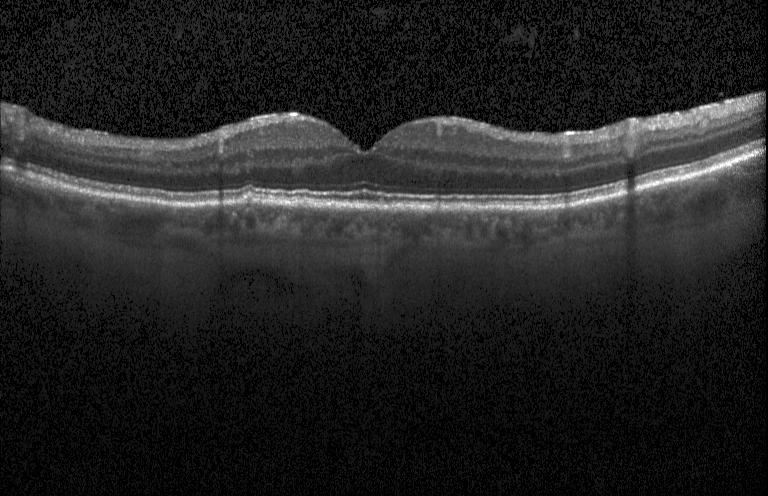 Finding: sub-RPE drusenoid deposits.